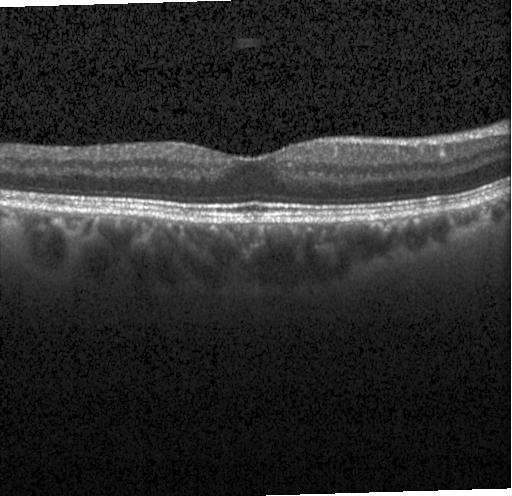 OCT B-scan.
No choroidal neovascularization, no diabetic macular edema, and no drusen.